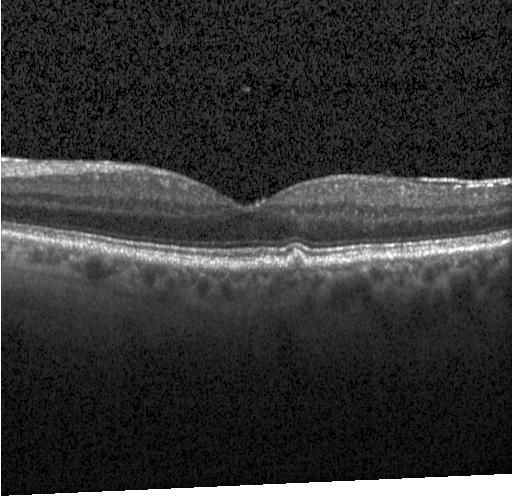
Spectral-domain OCT, macular scan, OCT B-scan, Heidelberg Spectralis OCT system
Diagnosis: drusen.